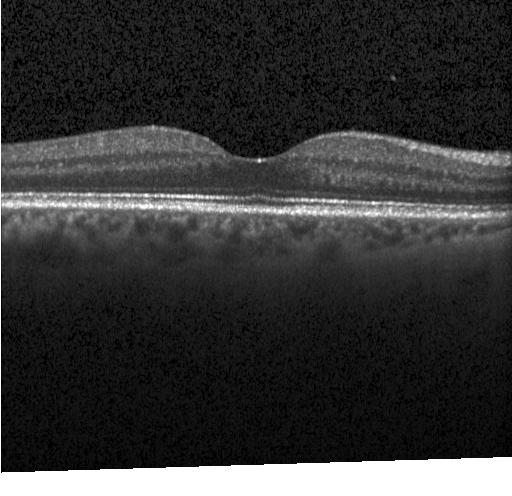 Optical coherence tomography B-scan; centered on the fovea. Diagnosis: no CNV, DME, or drusen.